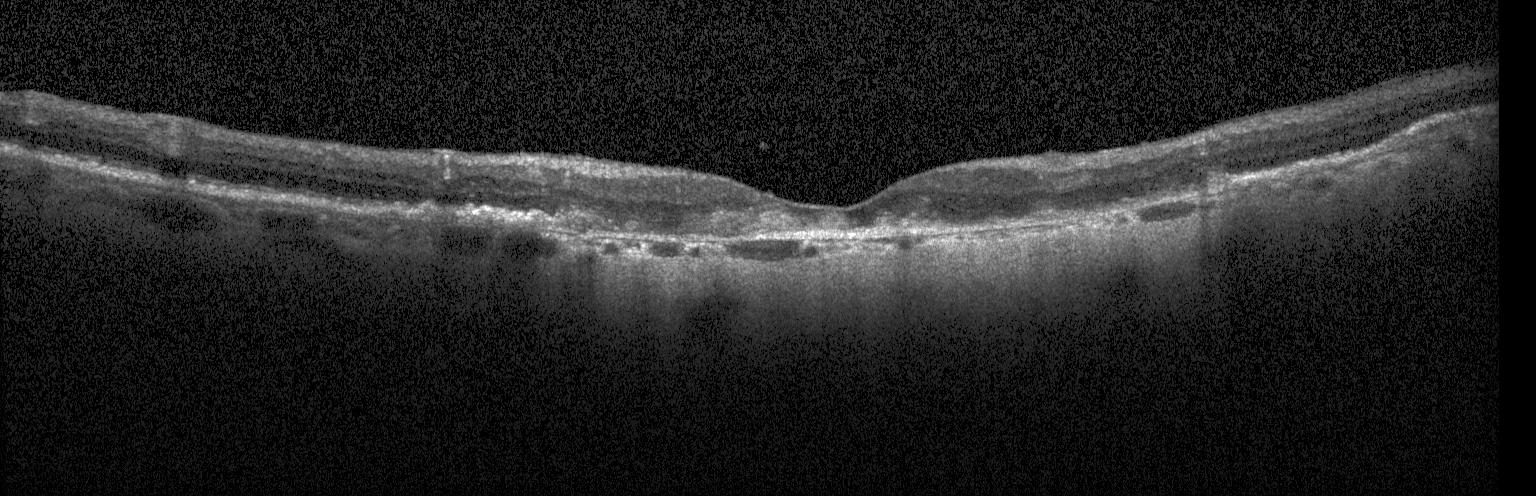 Dx: choroidal neovascularization (CNV).